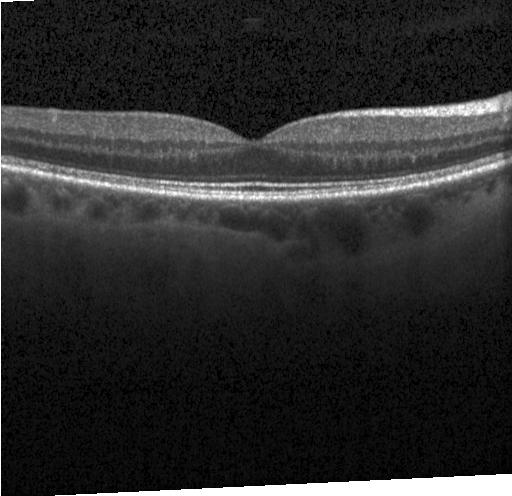
Optical coherence tomography scan · macular scan · spectral-domain OCT
Finding: neither CNV, DME, nor drusen.